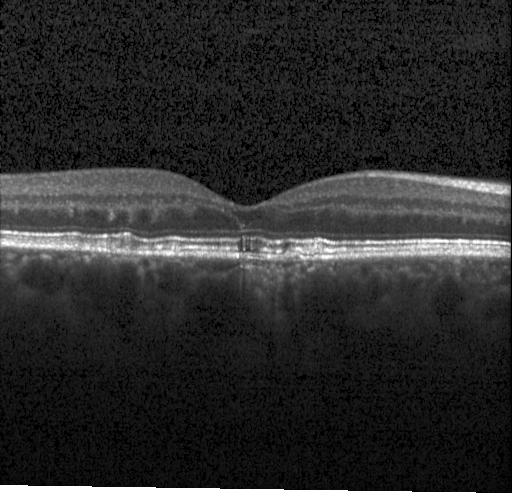
Through the macula · retinal OCT B-scan. This B-scan demonstrates drusen.